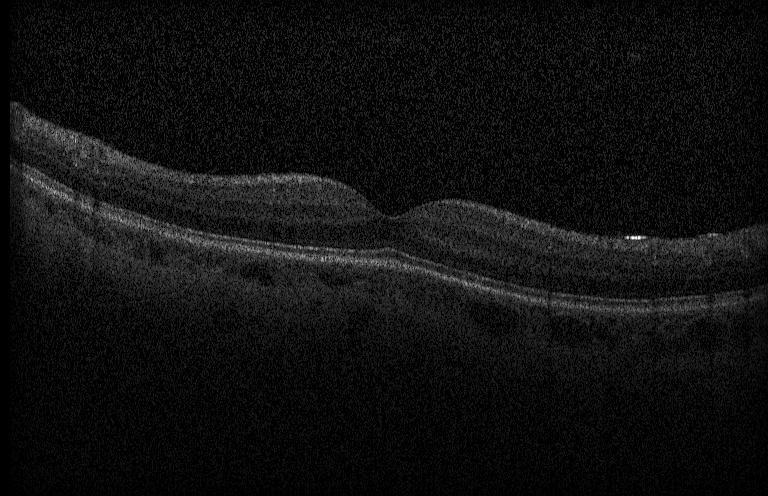

Diagnosis: neither CNV, DME, nor drusen.